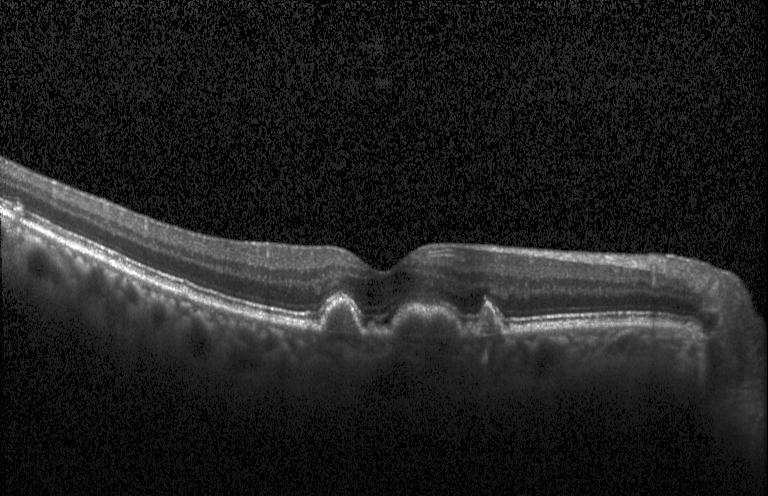
OCT B-scan; centered on the fovea
Assessment: multiple drusen.